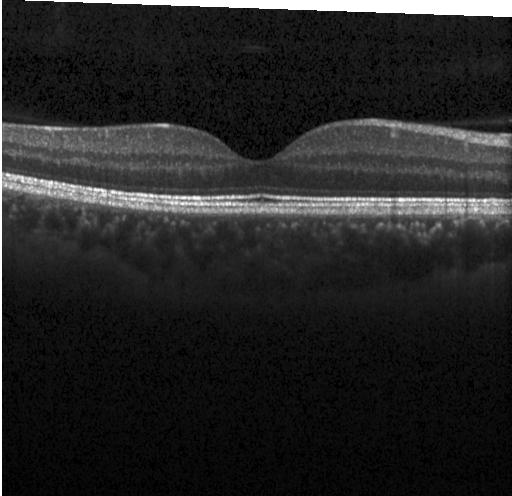
Spectral-domain optical coherence tomography. Retinal OCT B-scan. Instrument: Heidelberg Spectralis
The scan shows no CNV, DME, or drusen.